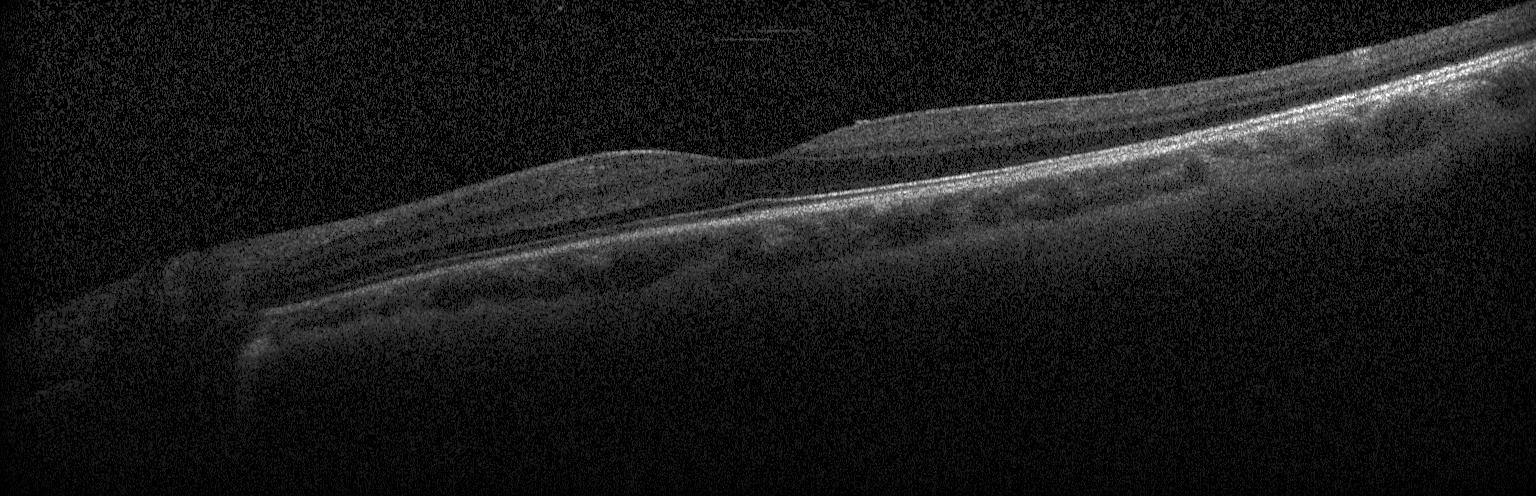

Retinal OCT B-scan. OCT finding: no choroidal neovascularization, diabetic macular edema, or drusen.